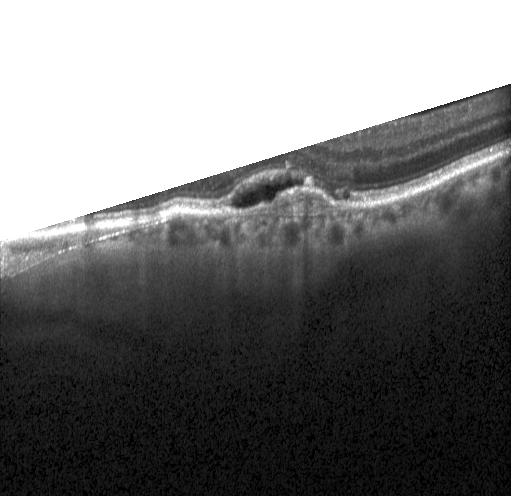
Finding: CNV.